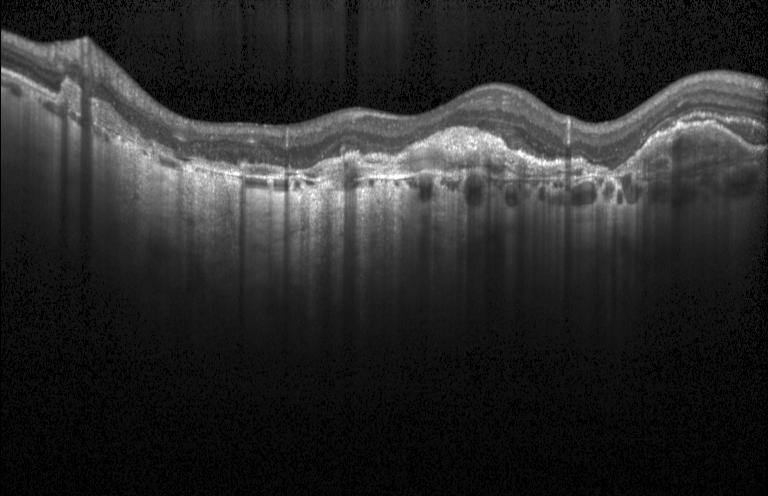 Optical coherence tomography B-scan · fovea-centered.
Choroidal neovascularization (CNV).